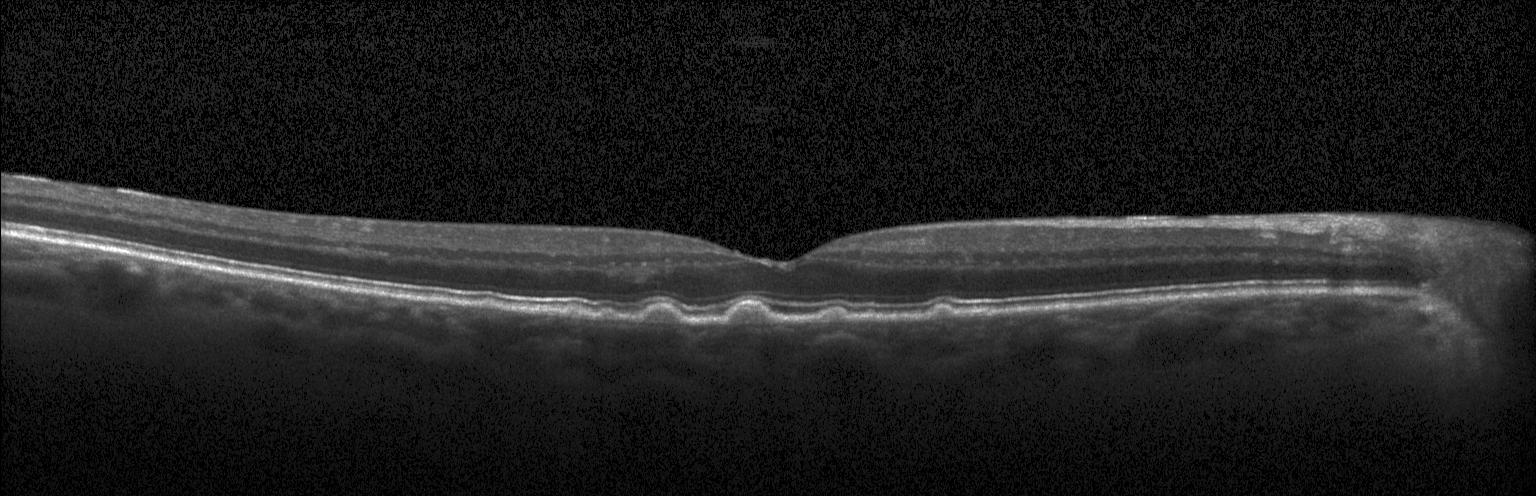
Horizontal scan through the fovea · optical coherence tomography B-scan. Macular OCT: sub-RPE drusenoid deposits.